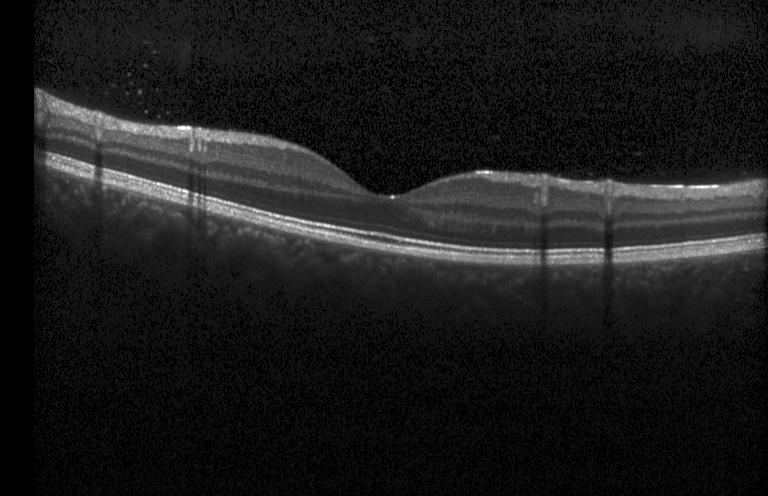

Macular OCT: no choroidal neovascularization, diabetic macular edema, or drusen.